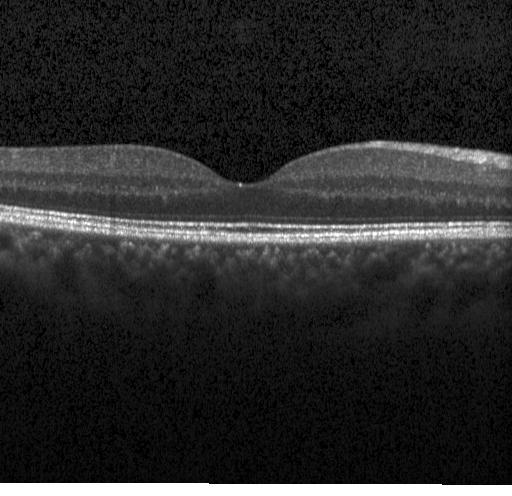 Retinal OCT cross-section showing neither choroidal neovascularization, diabetic macular edema, nor drusen.